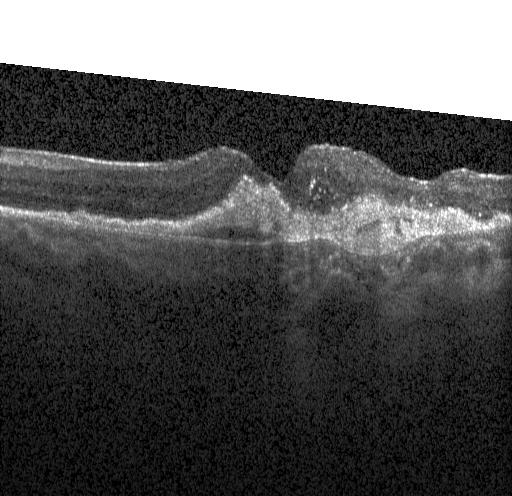

Optical coherence tomography scan
A choroidal neovascular membrane.